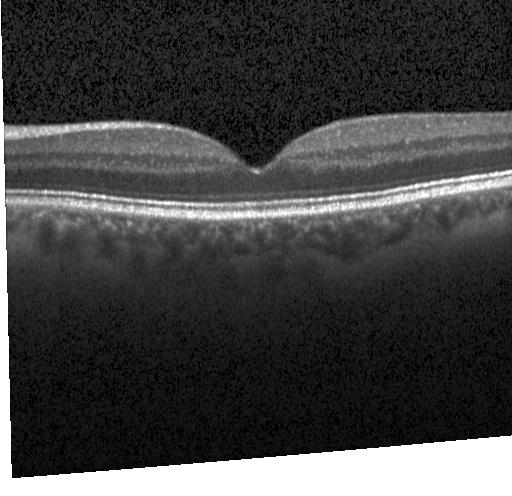
Centered on the fovea · optical coherence tomography B-scan · spectral-domain OCT — Neither CNV, DME, nor drusen.